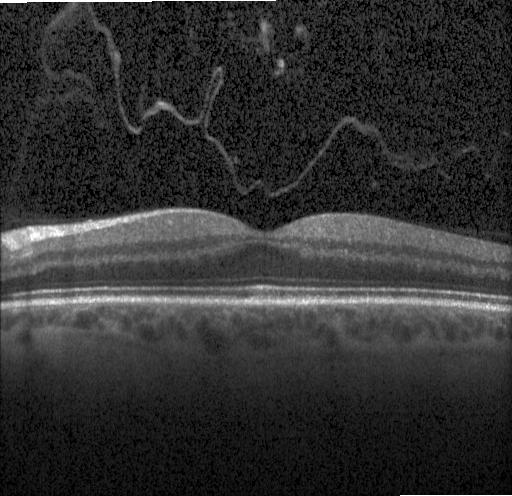

Retinal OCT B-scan; Heidelberg Spectralis; through the macula — This B-scan demonstrates no CNV, no DME, and no drusen.